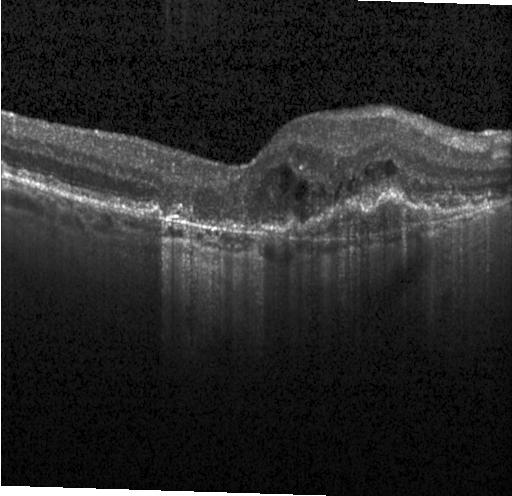
Spectral-domain optical coherence tomography · fovea-centered · optical coherence tomography scan
Finding: choroidal neovascularization.